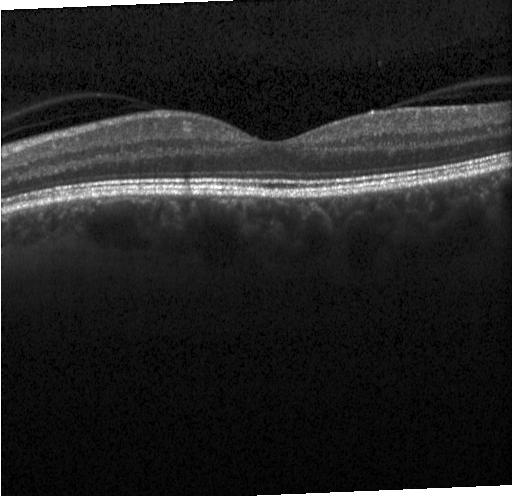
Horizontal scan through the fovea, retinal OCT cross-section
Impression: no evidence of choroidal neovascularization, diabetic macular edema, or drusen.